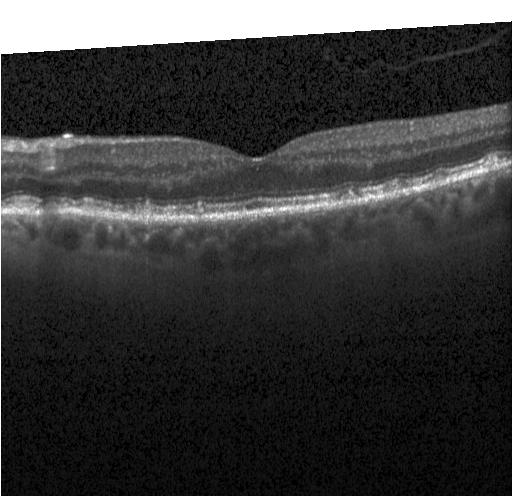
Finding: drusen.